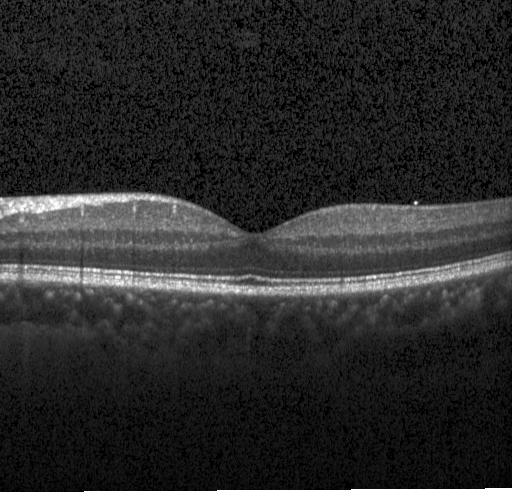 SD-OCT, retinal OCT cross-section, instrument: Heidelberg Spectralis, horizontal scan through the fovea.
Diagnosis: no evidence of choroidal neovascularization, diabetic macular edema, or drusen.